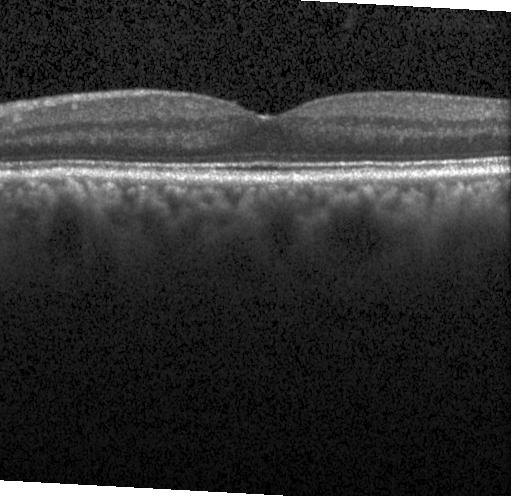

Retinal OCT cross-section.
Finding: neither choroidal neovascularization, diabetic macular edema, nor drusen.